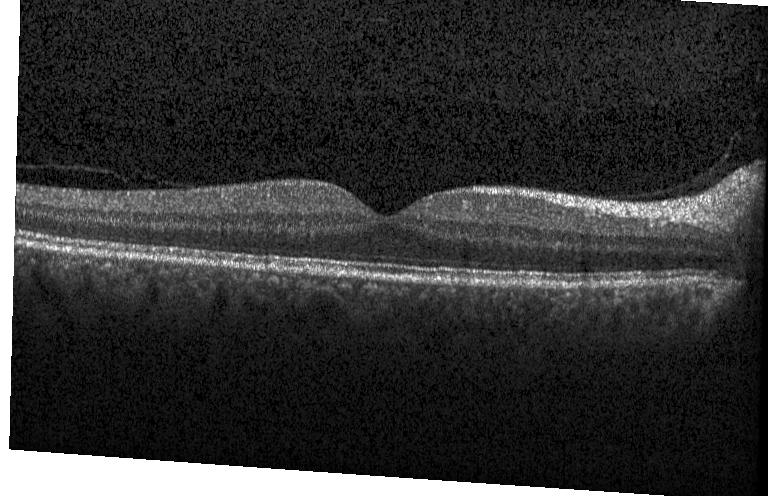 OCT scan showing no choroidal neovascularization, no diabetic macular edema, and no drusen.